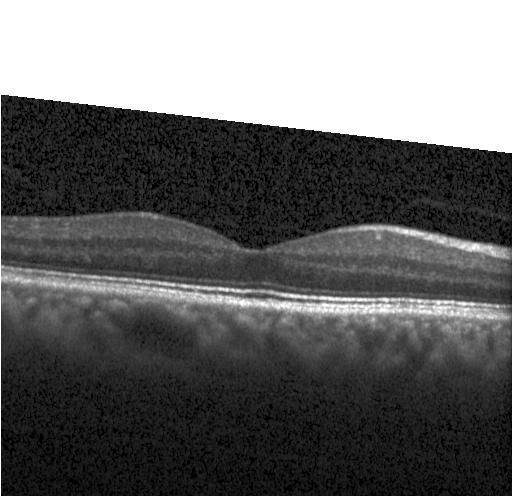

Heidelberg Spectralis OCT system; optical coherence tomography B-scan; centered on the fovea — Finding: no choroidal neovascularization, diabetic macular edema, or drusen.